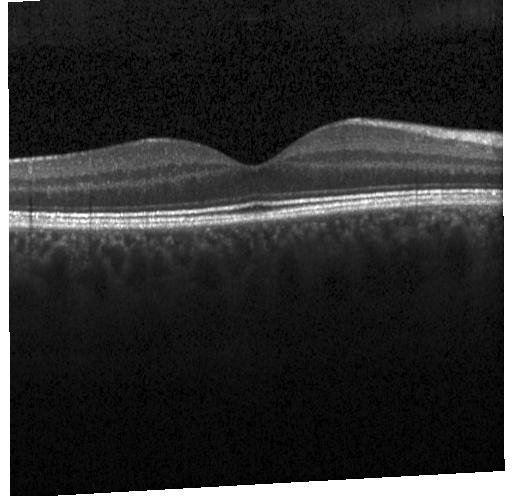

Dx: no choroidal neovascularization, diabetic macular edema, or drusen.